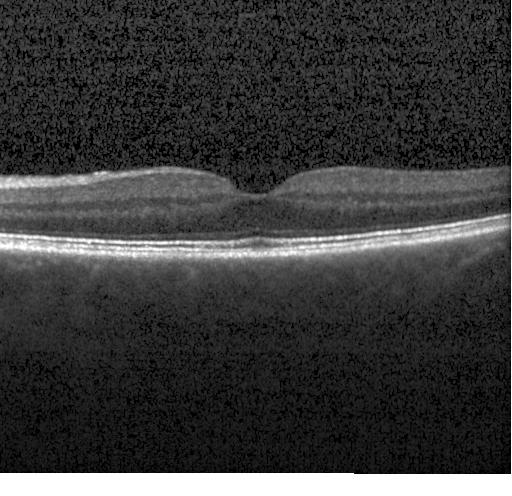 Finding: no choroidal neovascularization, diabetic macular edema, or drusen.